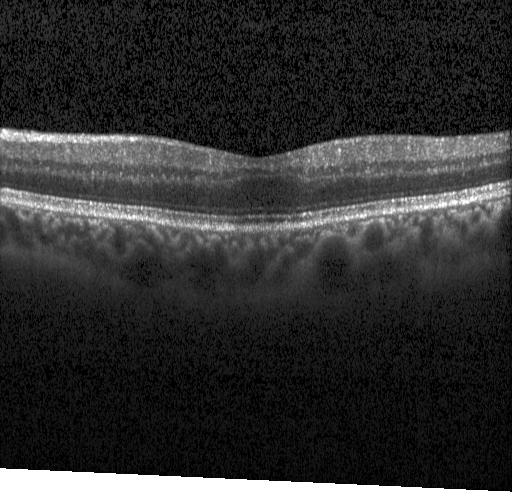
Spectral-domain OCT. OCT B-scan. Through the macula
Neither choroidal neovascularization, diabetic macular edema, nor drusen.